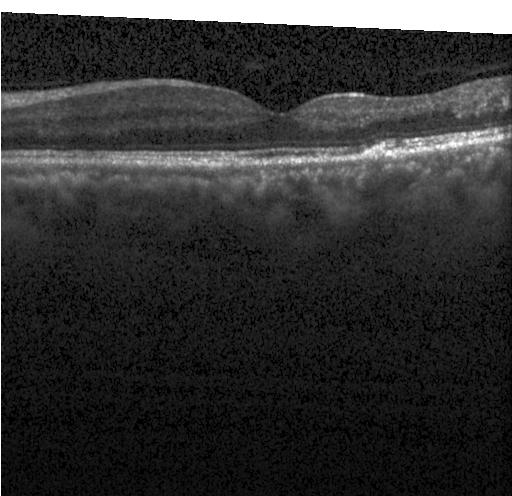 Assessment: drusen.